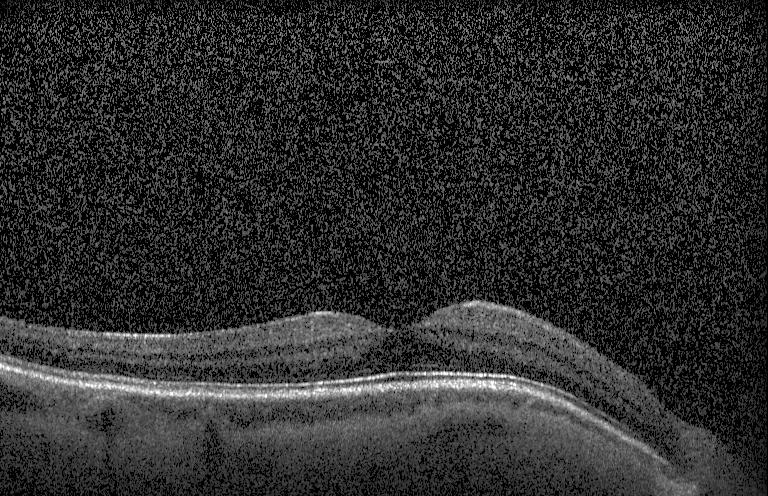

OCT B-scan · spectral-domain OCT · fovea-centered.
Diagnosis: no CNV, no DME, and no drusen.